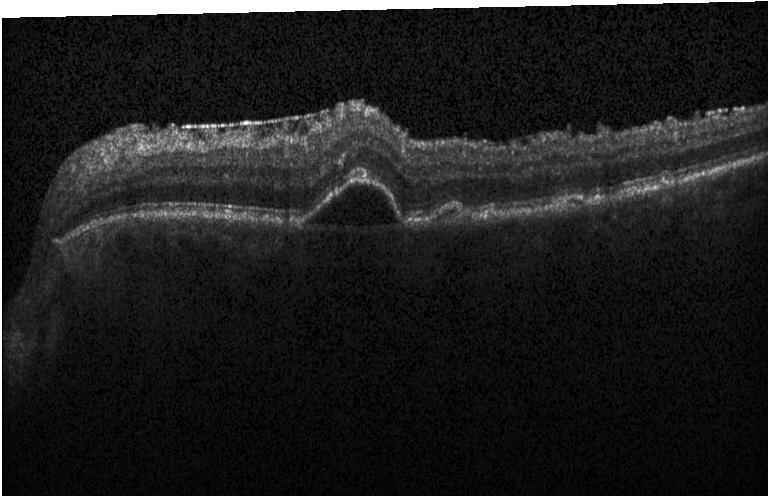 Centered on the fovea; retinal OCT B-scan. A choroidal neovascular membrane.